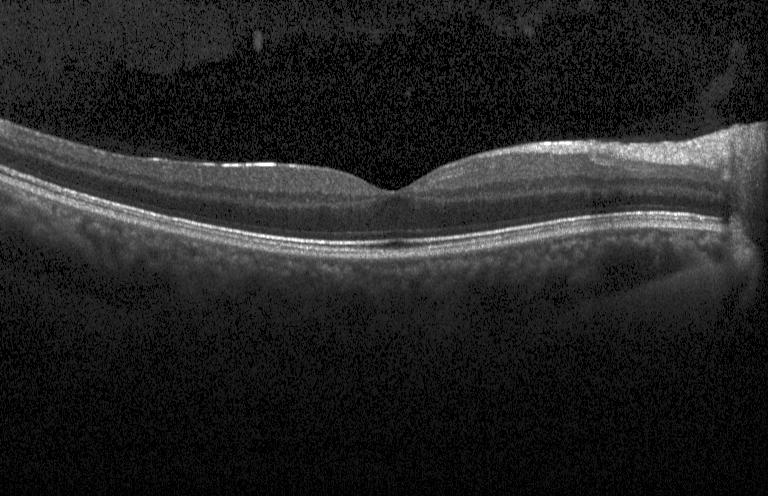
Spectral-domain optical coherence tomography · retinal OCT cross-section.
Impression: neither choroidal neovascularization, diabetic macular edema, nor drusen.